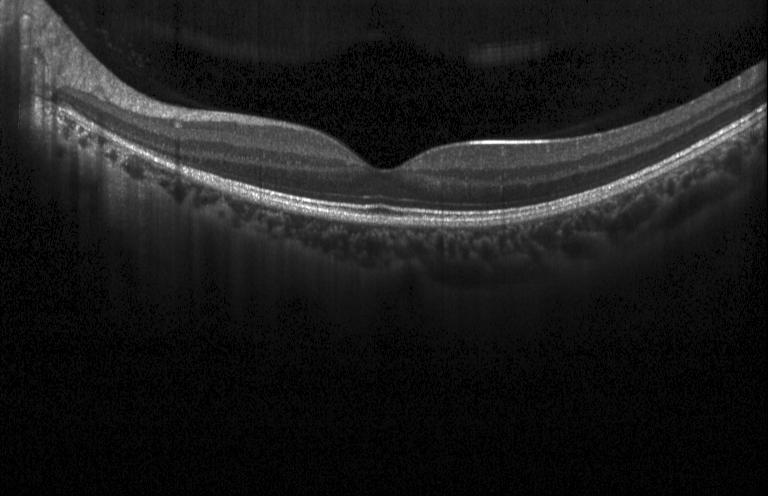
OCT finding: no evidence of choroidal neovascularization, diabetic macular edema, or drusen.